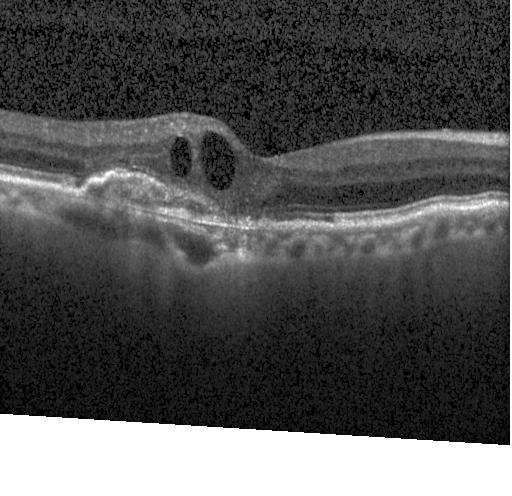

Heidelberg Spectralis. Retinal OCT B-scan
Macular OCT: CNV.